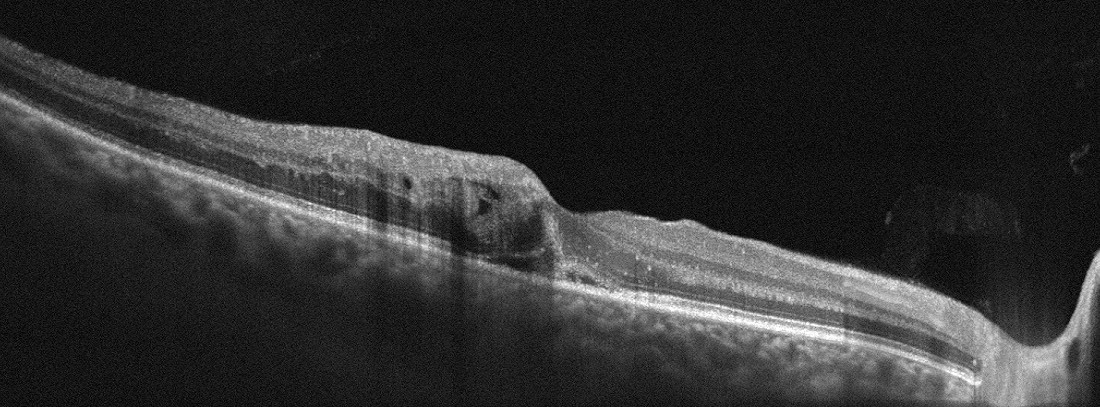
Acquired on an Optovue Avanti RTVue XR, fovea-centered, optical coherence tomography scan
Finding: retinal vein occlusion (RVO).